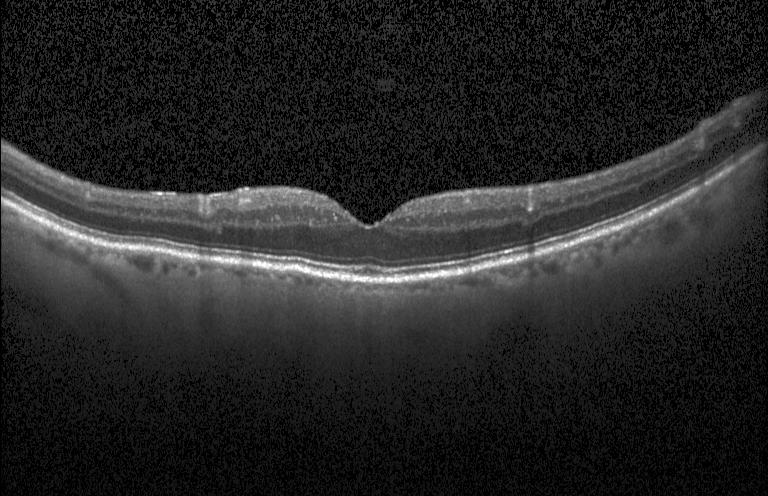
Diagnosis: no choroidal neovascularization, no diabetic macular edema, and no drusen.